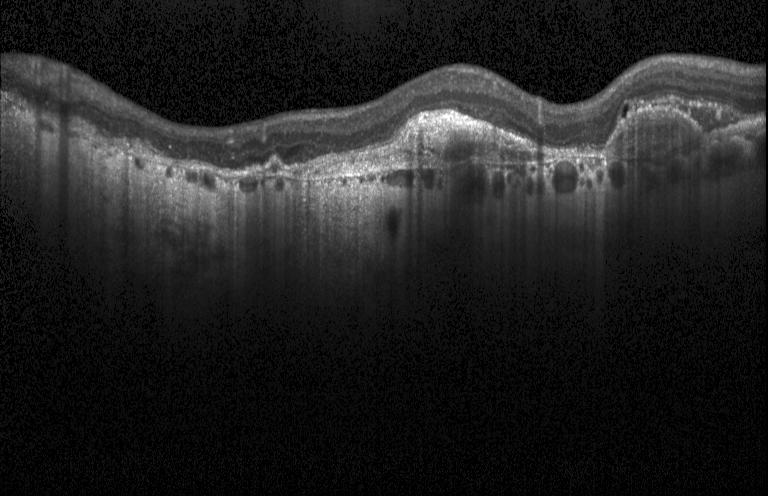 Retinal OCT B-scan
Dx: a choroidal neovascular membrane.